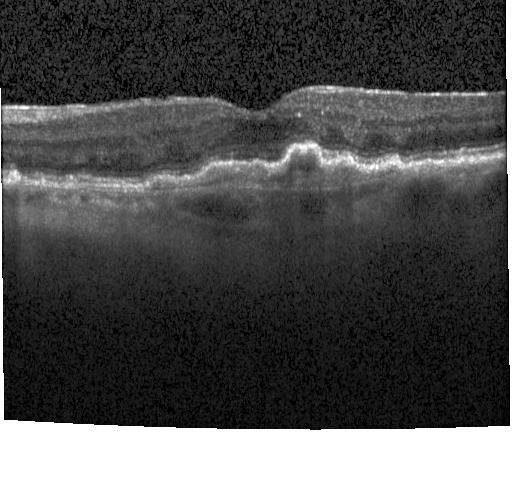 This B-scan demonstrates CNV.